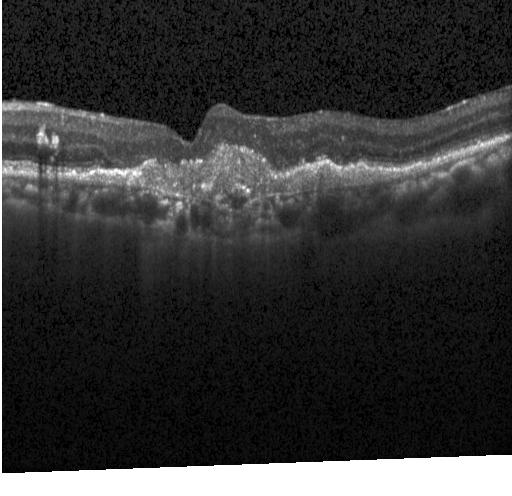 Instrument: Heidelberg Spectralis · retinal OCT B-scan · spectral-domain optical coherence tomography. The scan shows choroidal neovascularization.